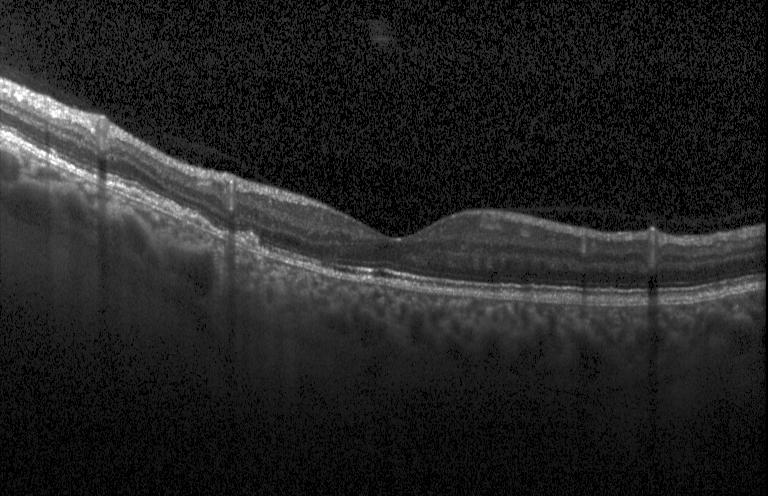 Spectral-domain OCT B-scan: CNV.